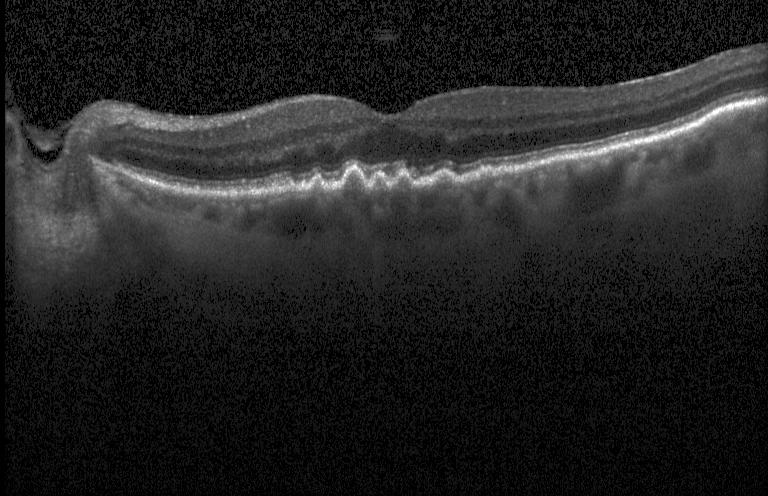

Heidelberg Spectralis. Spectral-domain OCT. Through the macula. OCT B-scan. Diagnosis: drusen.